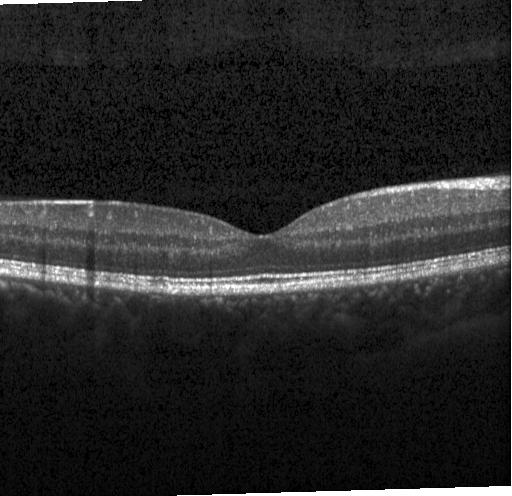
Spectral-domain OCT, retinal OCT B-scan
Impression: no evidence of CNV, DME, or drusen.